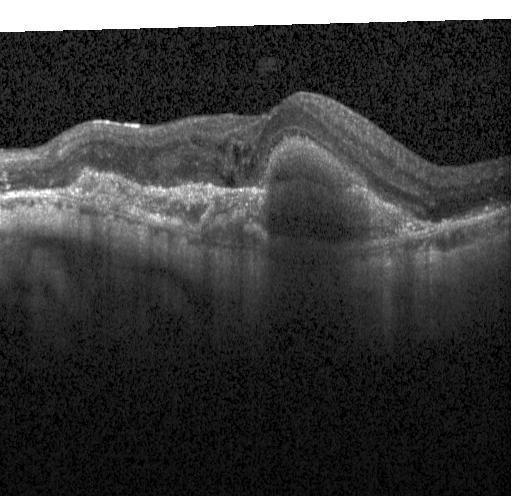 OCT line scan; spectral-domain OCT; through the macula; Heidelberg Spectralis — The scan shows choroidal neovascularization.